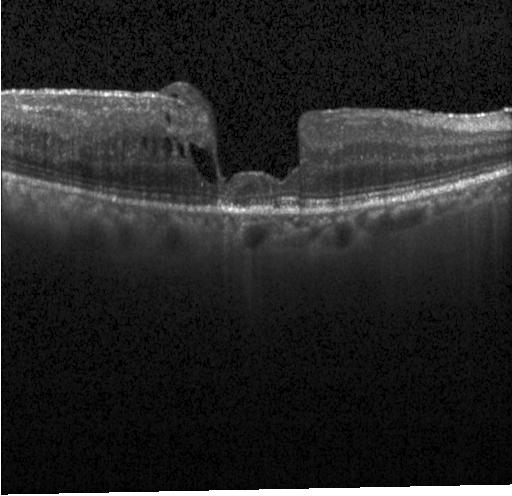 Retinal OCT cross-section showing diabetic macular edema.